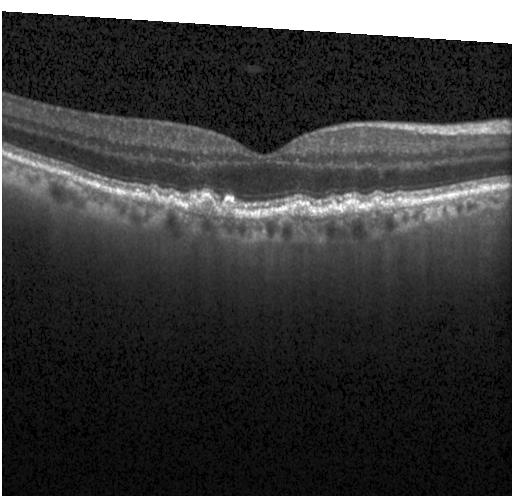

The scan shows drusen.